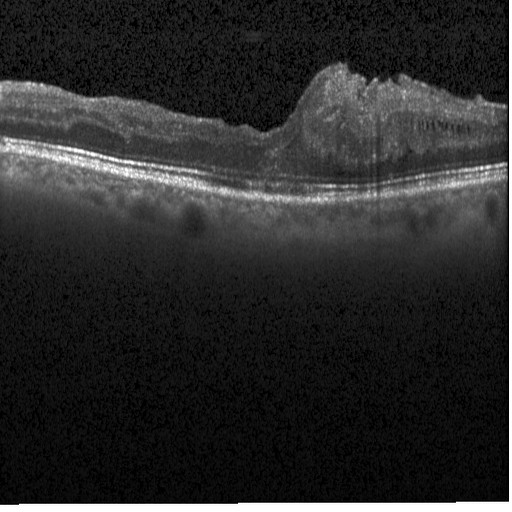 Diabetic macular edema.